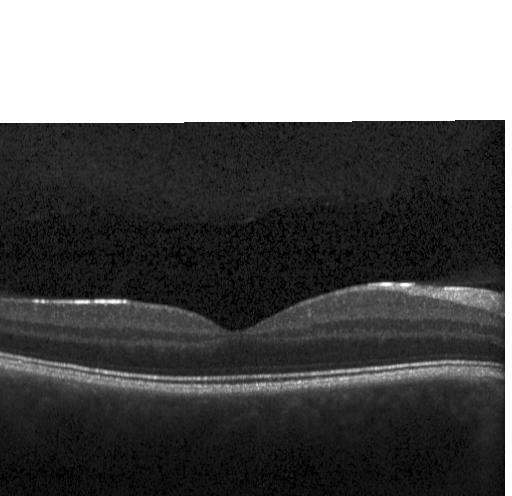
Assessment: no CNV, no DME, and no drusen.